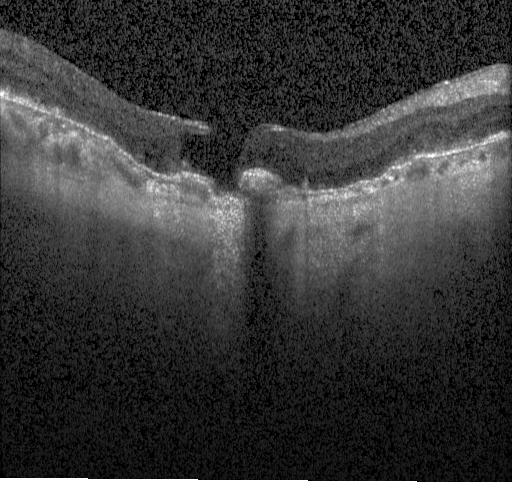

OCT line scan · fovea-centered · SD-OCT. OCT finding: a choroidal neovascular membrane.